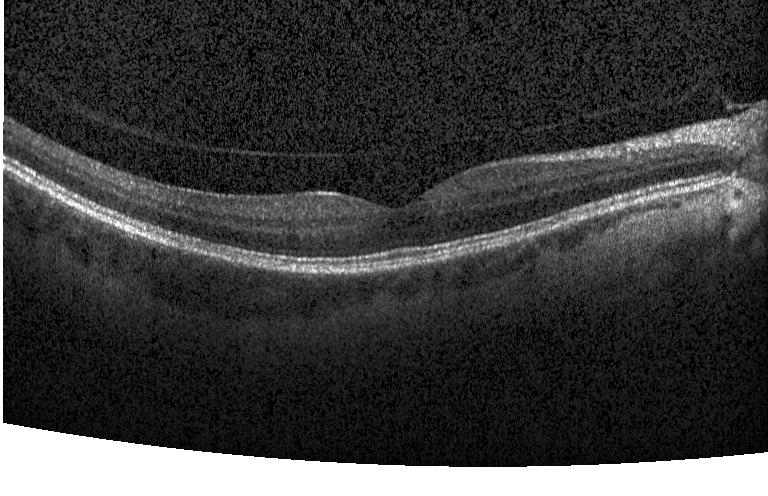 Fovea-centered; optical coherence tomography B-scan; spectral-domain optical coherence tomography.
OCT finding: no evidence of choroidal neovascularization, diabetic macular edema, or drusen.